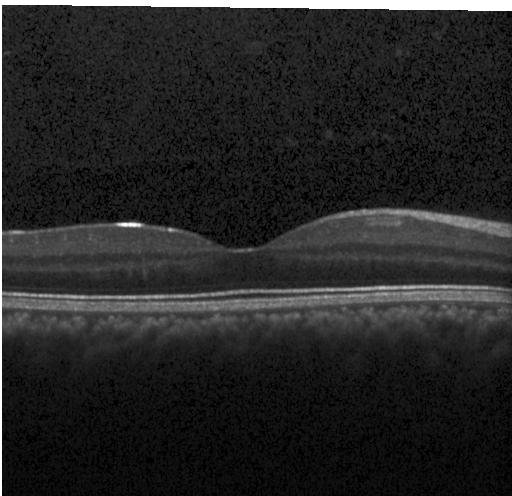
Diagnosis: no CNV, DME, or drusen.